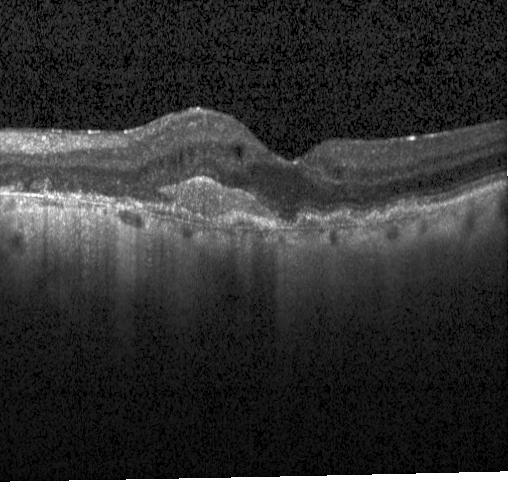
Fovea-centered, optical coherence tomography scan — The scan shows a choroidal neovascular membrane.